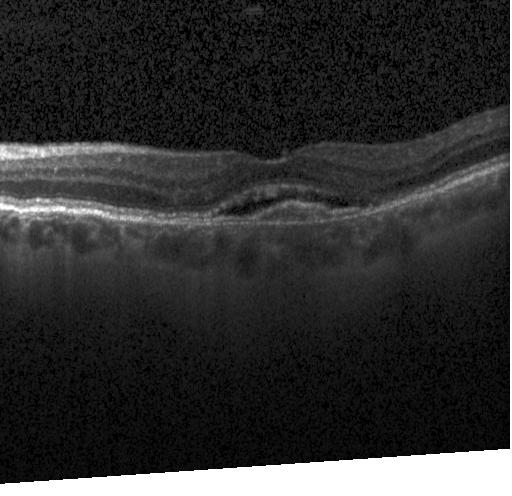

SD-OCT, retinal OCT cross-section
Macular OCT: choroidal neovascularization (CNV).